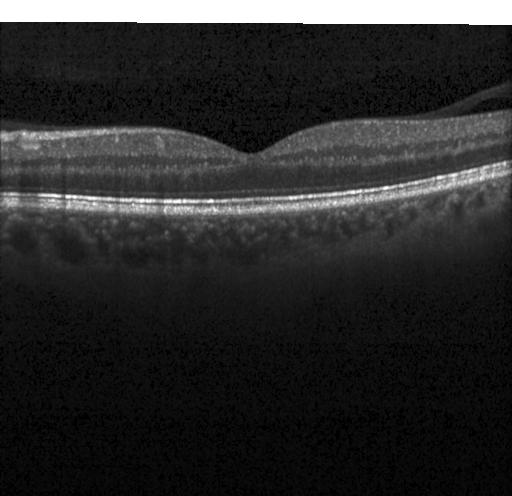

OCT line scan. Macular scan
Assessment: no CNV, no DME, and no drusen.